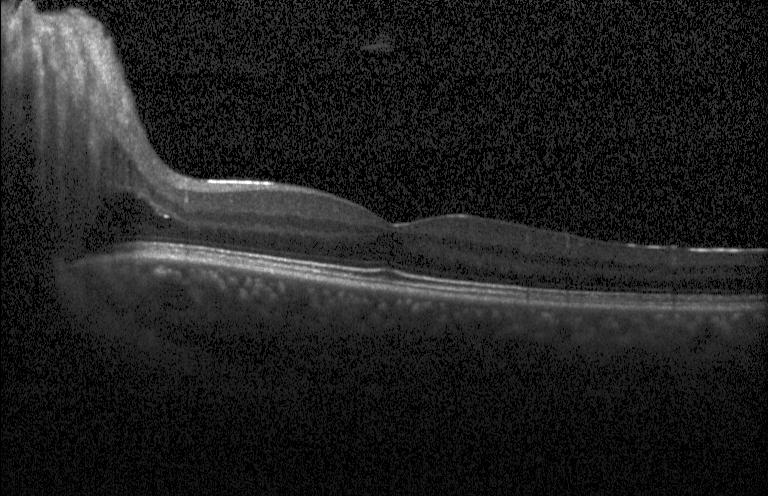
Retinal OCT cross-section · Heidelberg Spectralis · horizontal scan through the fovea · SD-OCT — Impression: no choroidal neovascularization, no diabetic macular edema, and no drusen.